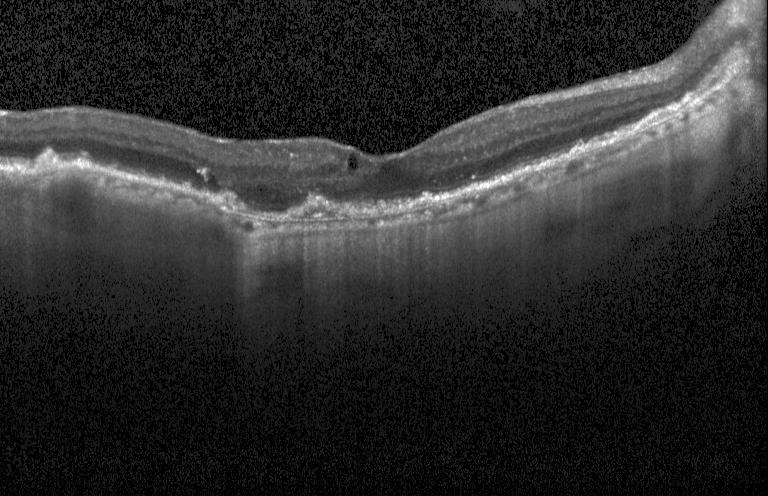 Optical coherence tomography B-scan.
A choroidal neovascular membrane.